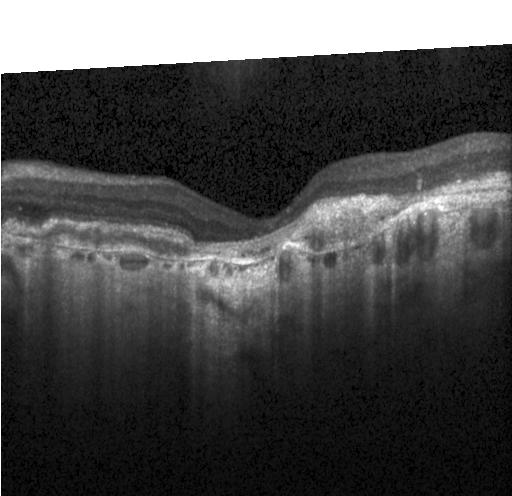
OCT B-scan showing a choroidal neovascular membrane.